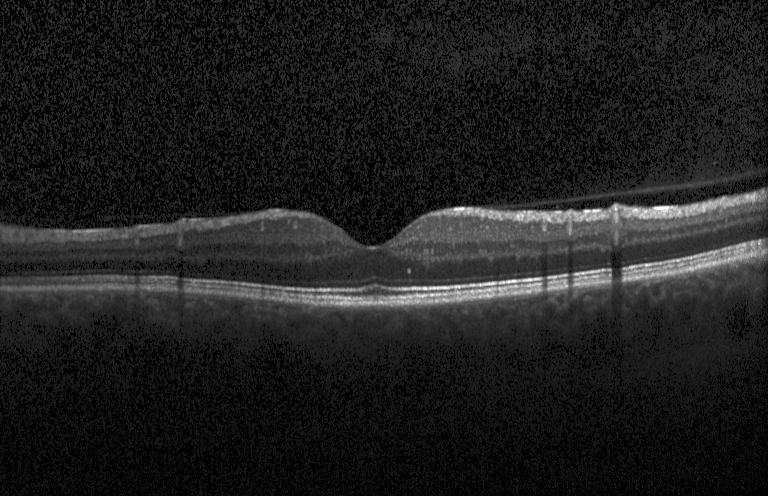
OCT line scan
Finding: no choroidal neovascularization, no diabetic macular edema, and no drusen.